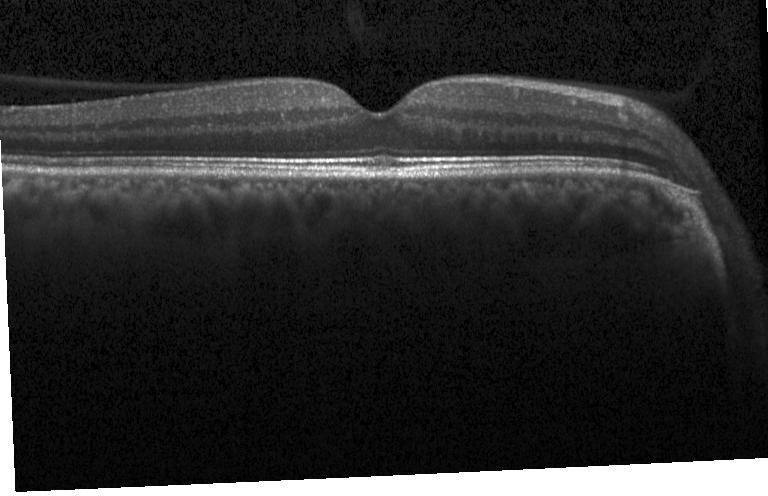
Finding: neither choroidal neovascularization, diabetic macular edema, nor drusen.